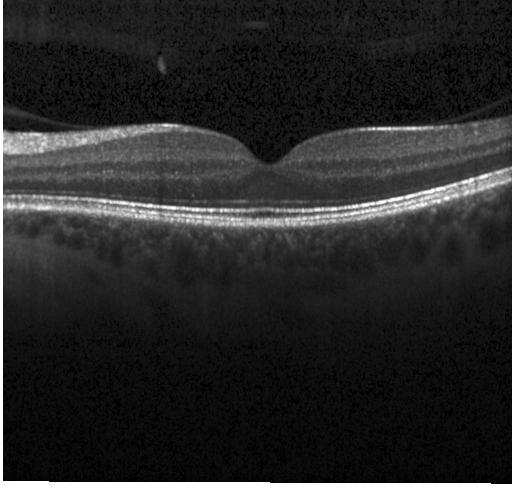 Retinal OCT cross-section, acquired on a Heidelberg Spectralis — Macular OCT: neither choroidal neovascularization, diabetic macular edema, nor drusen.